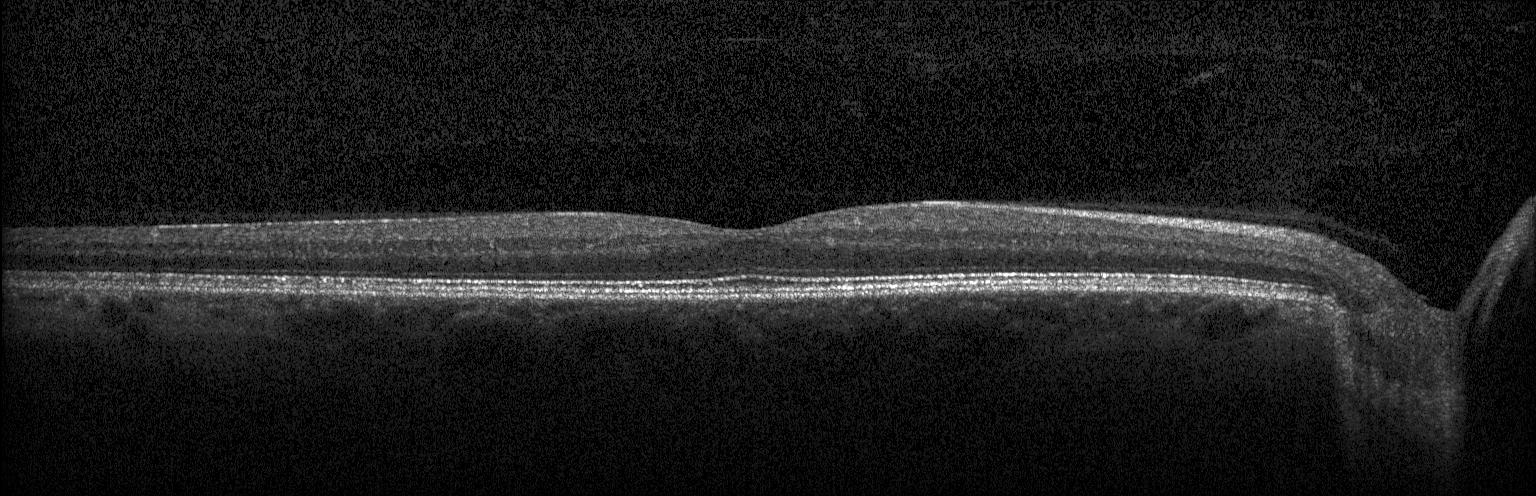

OCT line scan
Finding: no CNV, no DME, and no drusen.